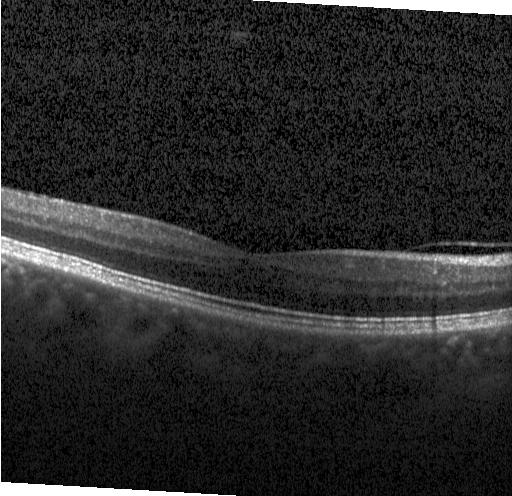

Spectral-domain OCT; fovea-centered; OCT line scan
Finding: no choroidal neovascularization, diabetic macular edema, or drusen.